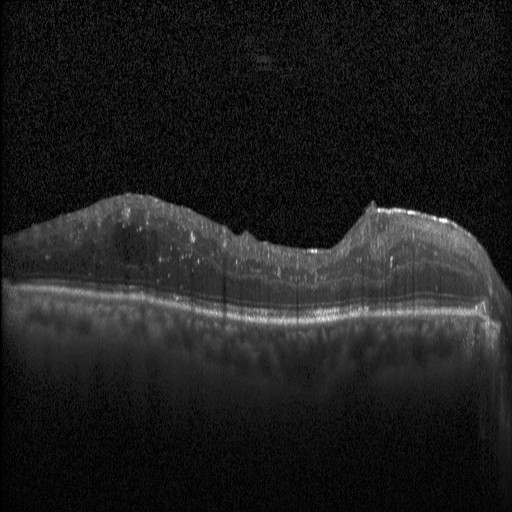

Retinal OCT B-scan — Macular OCT: diabetic macular edema.